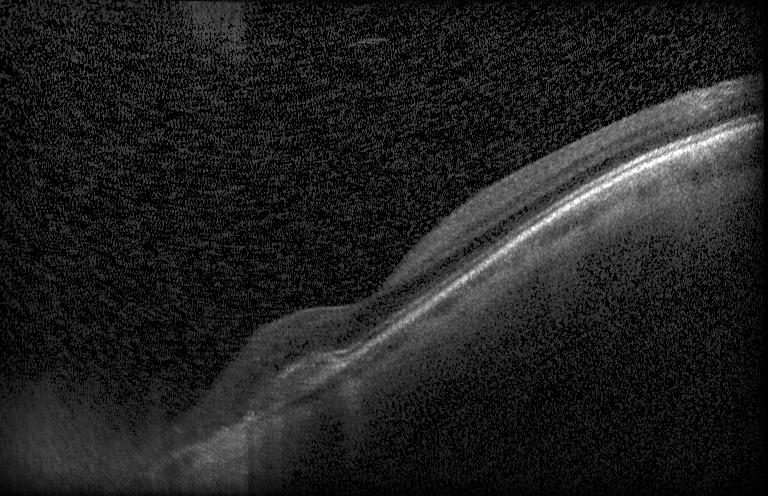 Diagnosis: a choroidal neovascular membrane.